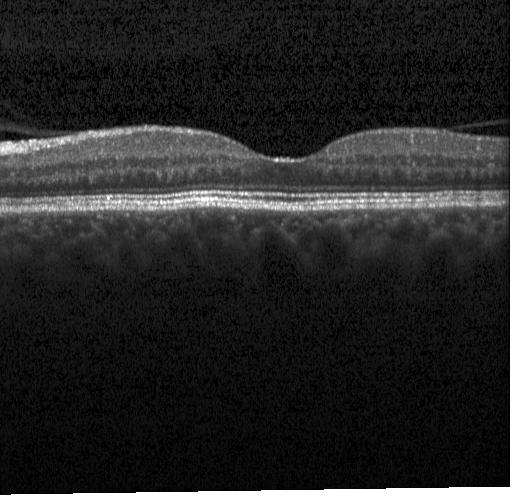

Impression: neither choroidal neovascularization, diabetic macular edema, nor drusen.